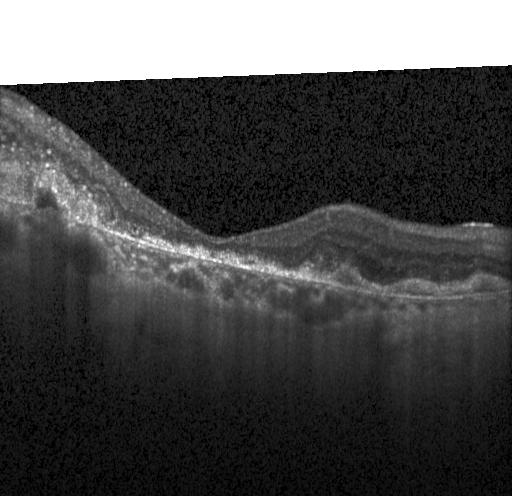

Retinal OCT B-scan; spectral-domain OCT; horizontal scan through the fovea. Finding: a choroidal neovascular membrane.